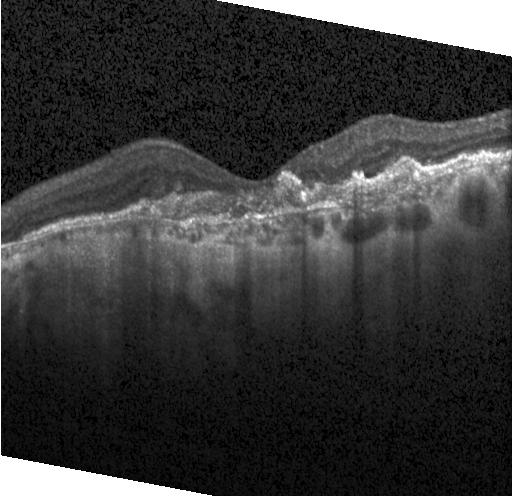

Heidelberg Spectralis; SD-OCT; horizontal scan through the fovea; retinal OCT cross-section — Macular OCT: a choroidal neovascular membrane.